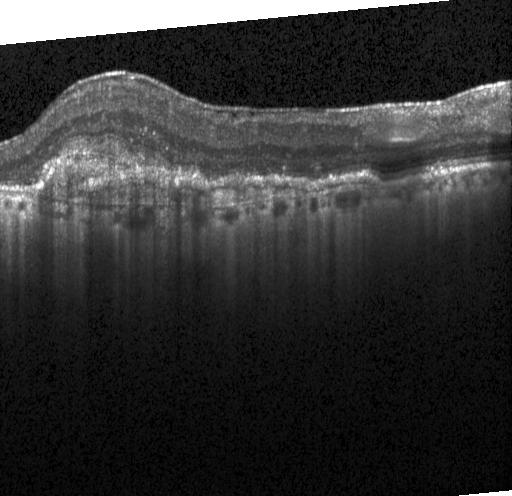
Retinal OCT B-scan — Impression: a choroidal neovascular membrane.